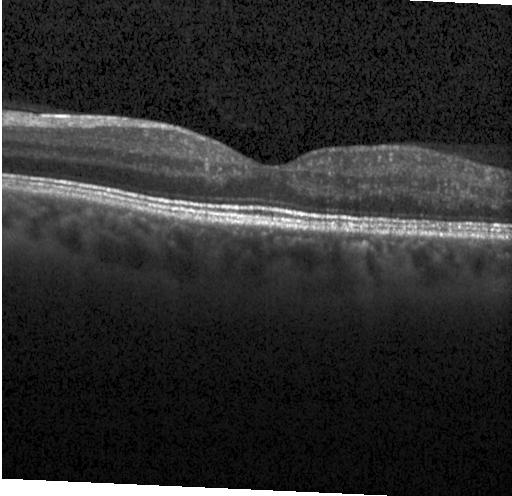
Diagnosis: no CNV, DME, or drusen.